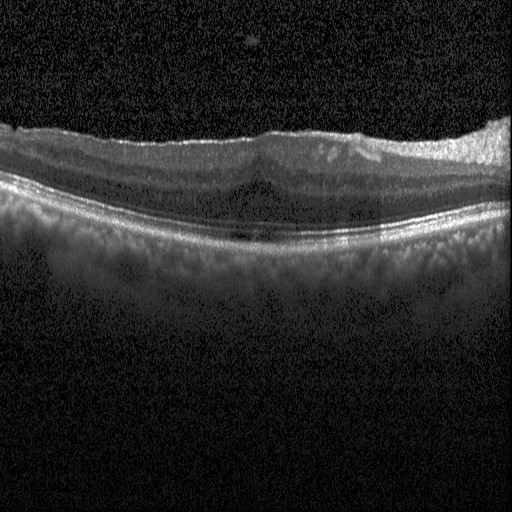

Acquired on a Heidelberg Spectralis. Retinal OCT cross-section.
Impression: DME.